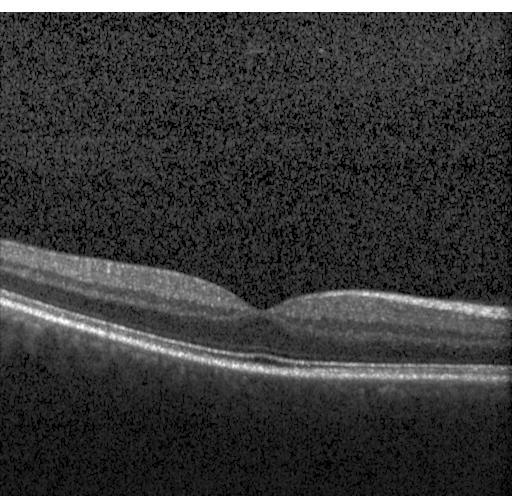 Acquired on a Heidelberg Spectralis · retinal OCT cross-section · spectral-domain OCT · horizontal scan through the fovea — The scan shows no choroidal neovascularization, diabetic macular edema, or drusen.